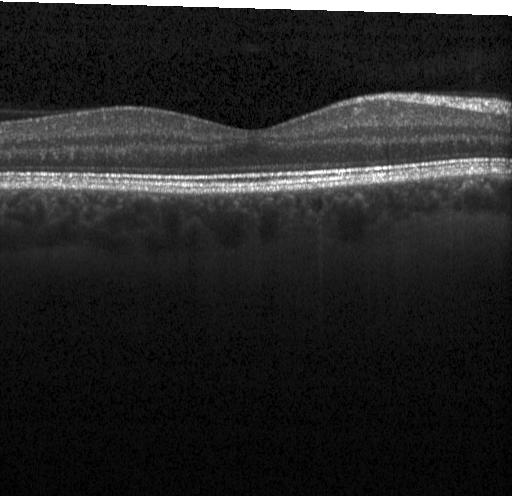
Spectral-domain OCT B-scan: neither choroidal neovascularization, diabetic macular edema, nor drusen.